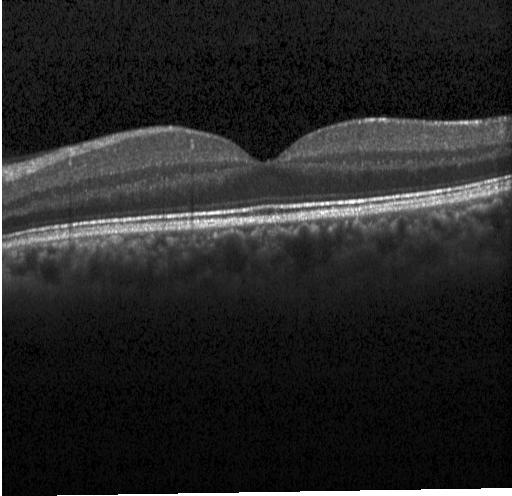

Impression: neither choroidal neovascularization, diabetic macular edema, nor drusen.